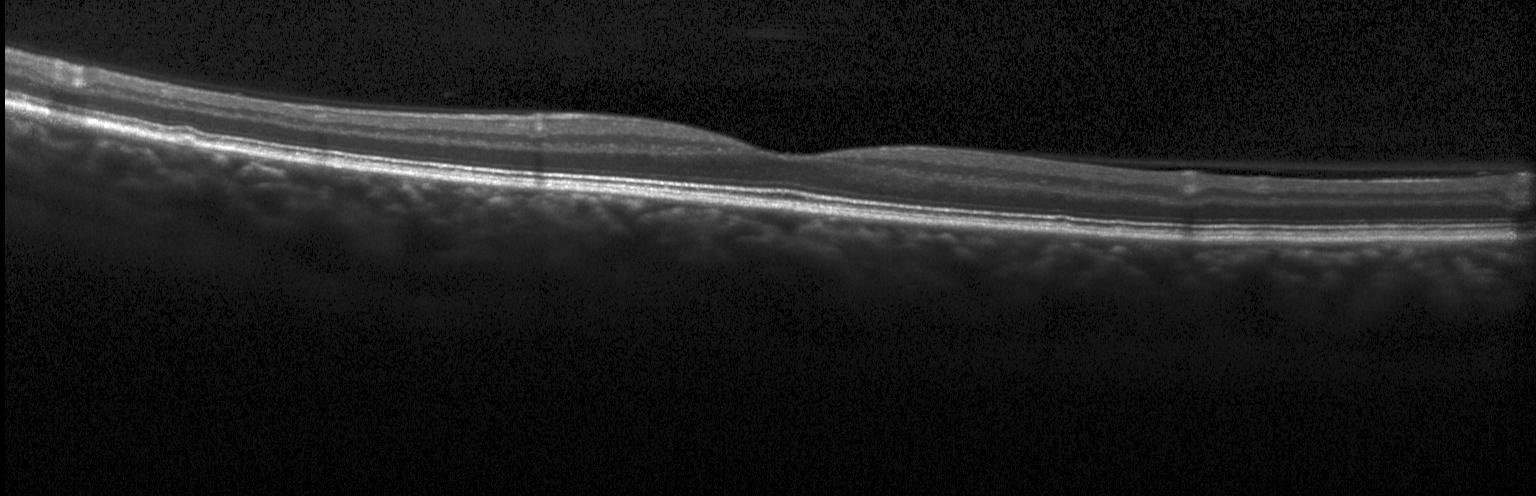 Retinal OCT B-scan, horizontal scan through the fovea.
Assessment: no evidence of choroidal neovascularization, diabetic macular edema, or drusen.